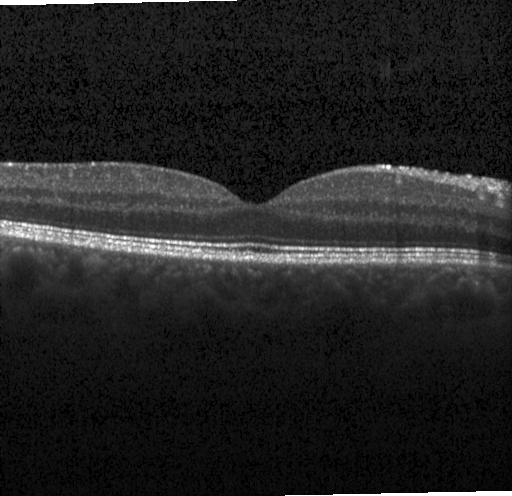 Impression: no choroidal neovascularization, diabetic macular edema, or drusen.